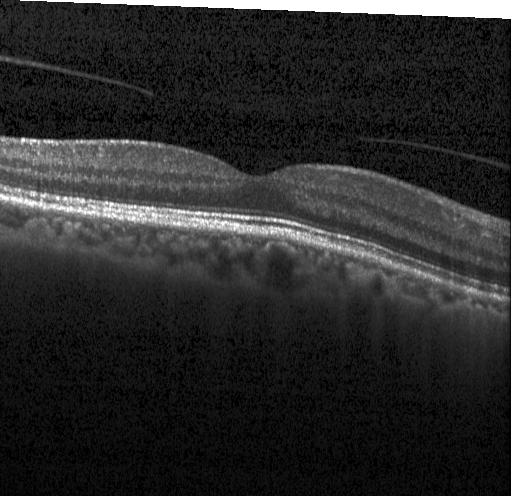

Retinal OCT B-scan.
Macular OCT: no choroidal neovascularization, no diabetic macular edema, and no drusen.